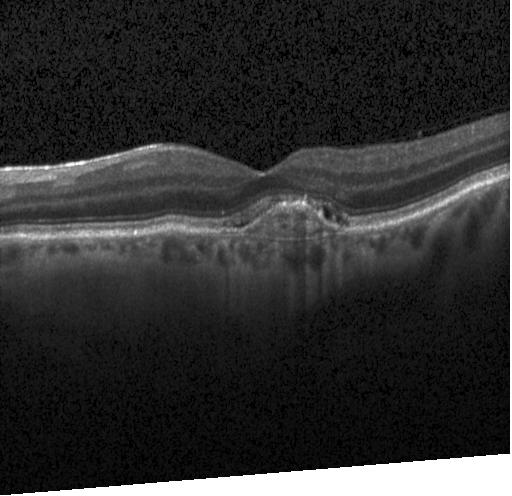
Assessment: a choroidal neovascular membrane.